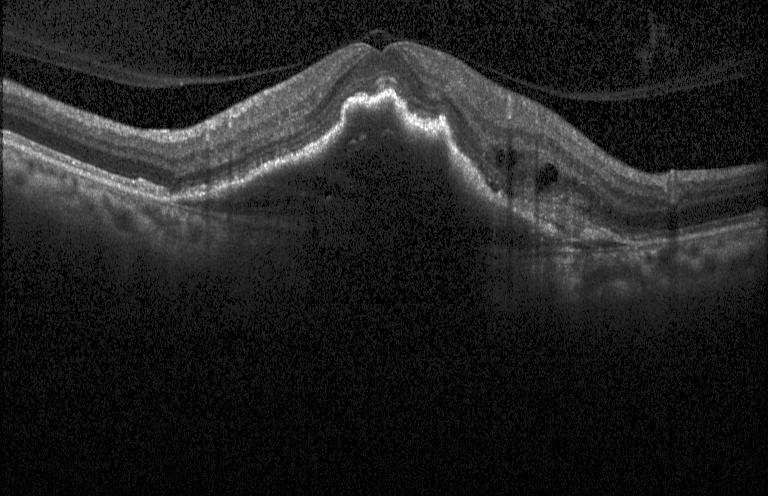

Finding: a choroidal neovascular membrane.